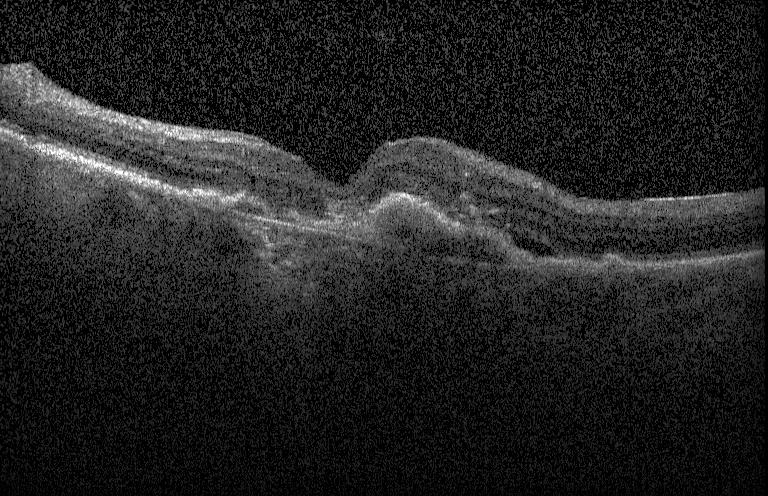 Dx: choroidal neovascularization (CNV).